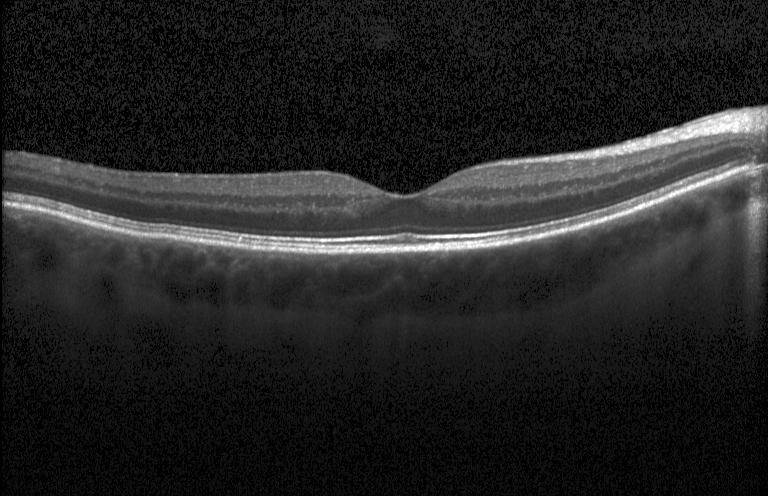

Retinal OCT B-scan. OCT finding: no CNV, DME, or drusen.